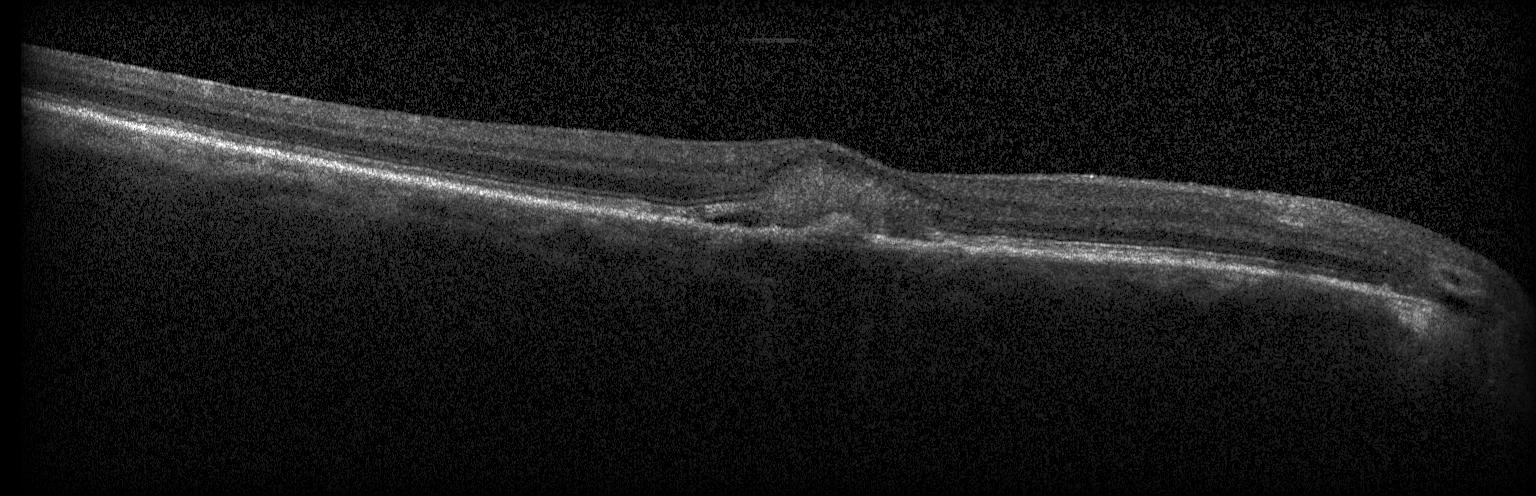
Dx: choroidal neovascularization (CNV).